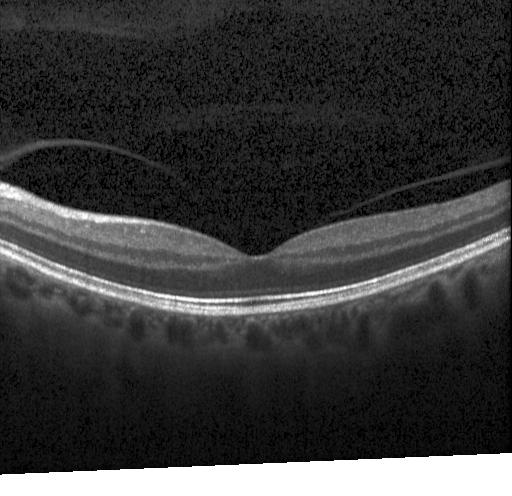
Diagnosis: neither choroidal neovascularization, diabetic macular edema, nor drusen.